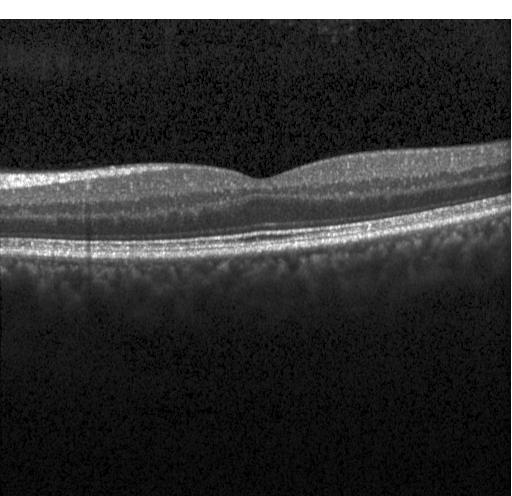
OCT line scan, fovea-centered, instrument: Heidelberg Spectralis
No evidence of choroidal neovascularization, diabetic macular edema, or drusen.